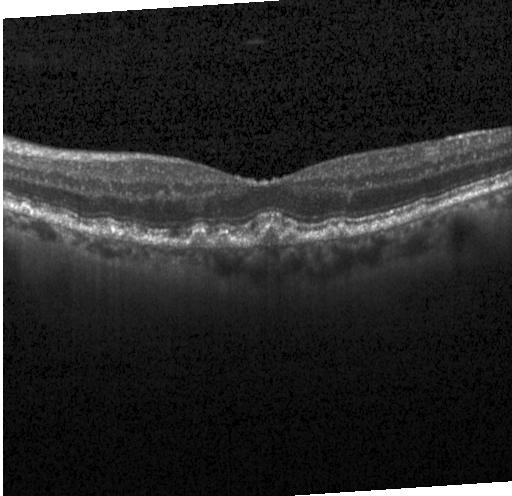

Through the macula. OCT line scan — Diagnosis: sub-RPE drusenoid deposits.